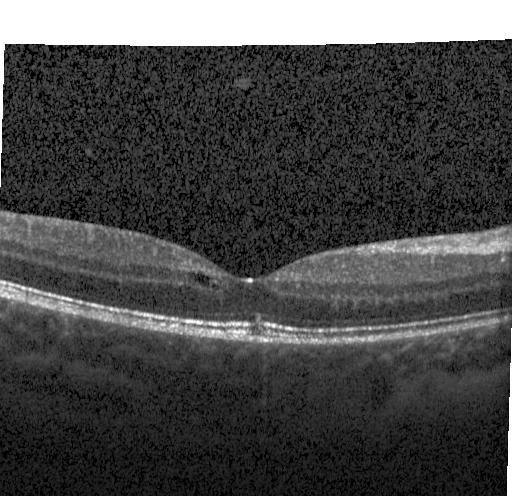
Acquired on a Heidelberg Spectralis · retinal OCT cross-section · spectral-domain OCT.
The scan shows diabetic macular edema.